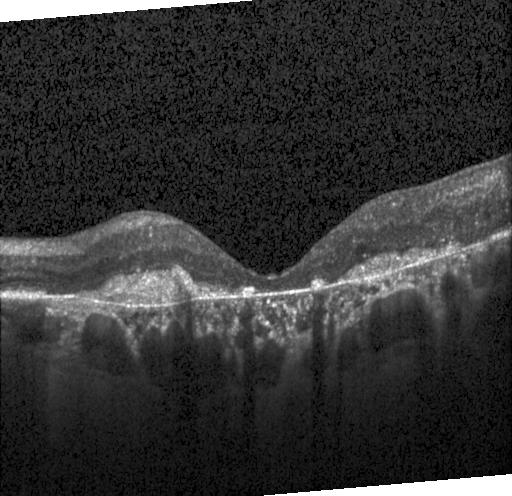

Macular OCT: a choroidal neovascular membrane.